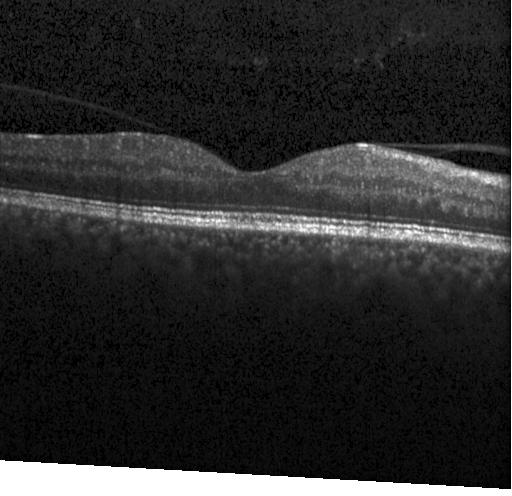

Impression: no evidence of choroidal neovascularization, diabetic macular edema, or drusen.